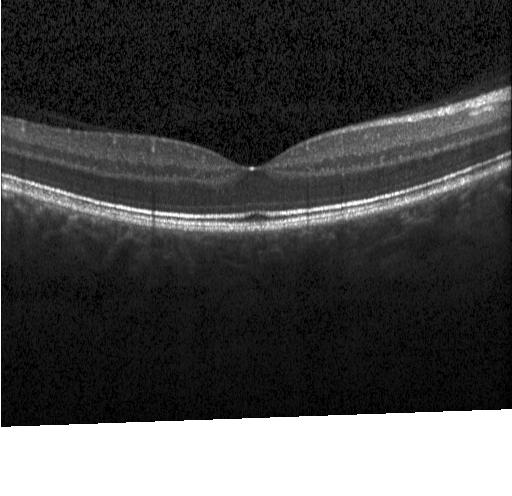 Fovea-centered; optical coherence tomography B-scan; instrument: Heidelberg Spectralis
Assessment: no CNV, no DME, and no drusen.